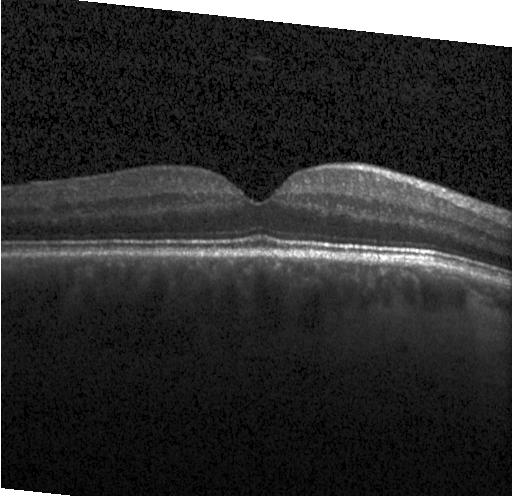

Retinal OCT B-scan
Diagnosis: no choroidal neovascularization, diabetic macular edema, or drusen.